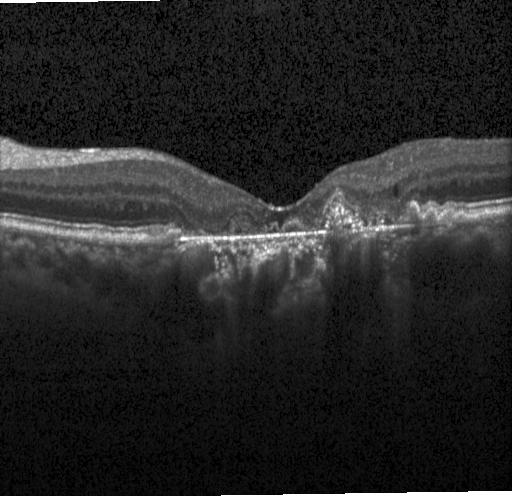 Optical coherence tomography B-scan · centered on the fovea. Assessment: choroidal neovascularization.